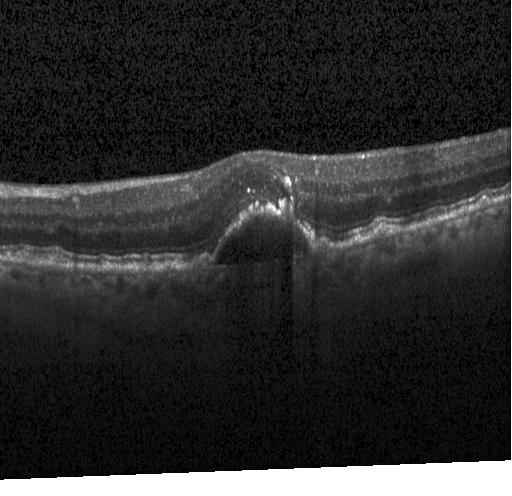
Acquired on a Heidelberg Spectralis; optical coherence tomography B-scan. This B-scan demonstrates CNV.